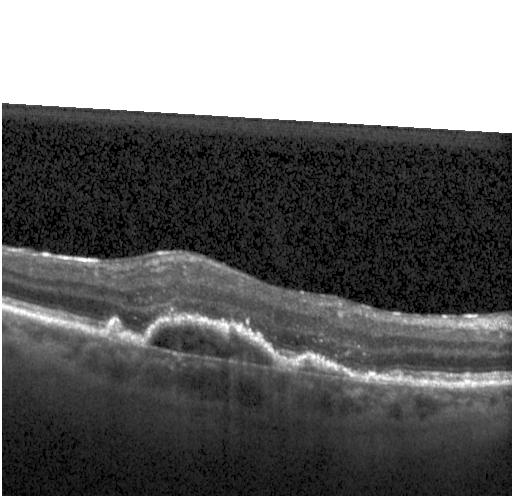
Dx: choroidal neovascularization (CNV).